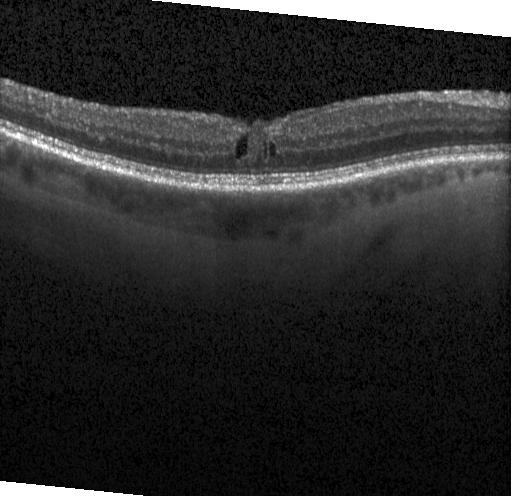 The scan shows diabetic macular edema (DME).